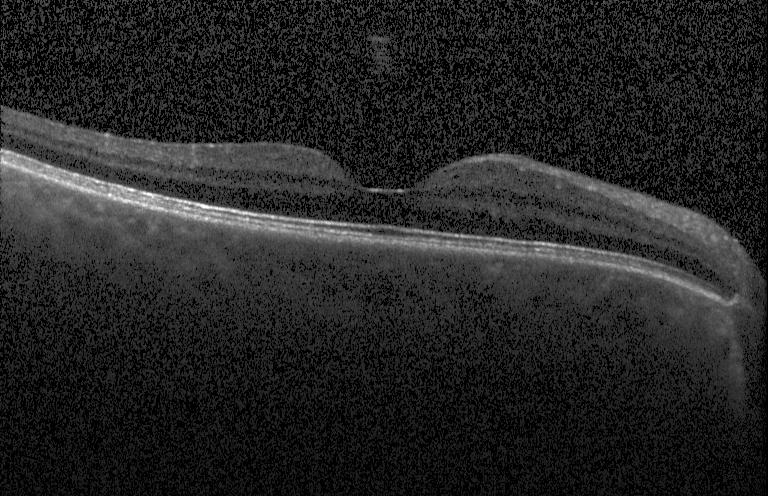

OCT B-scan.
This B-scan demonstrates neither CNV, DME, nor drusen.